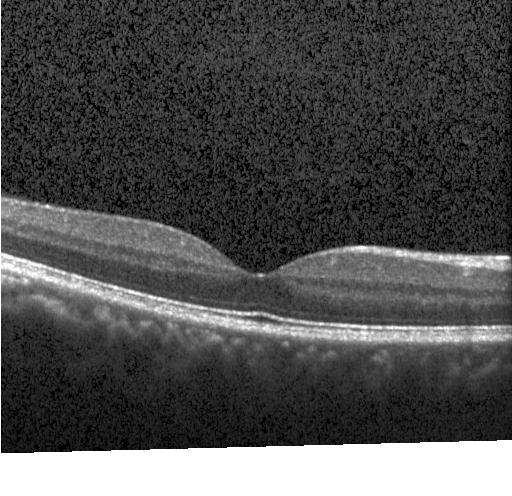
Macular scan; acquired on a Heidelberg Spectralis; SD-OCT; optical coherence tomography scan.
Dx: no choroidal neovascularization, diabetic macular edema, or drusen.